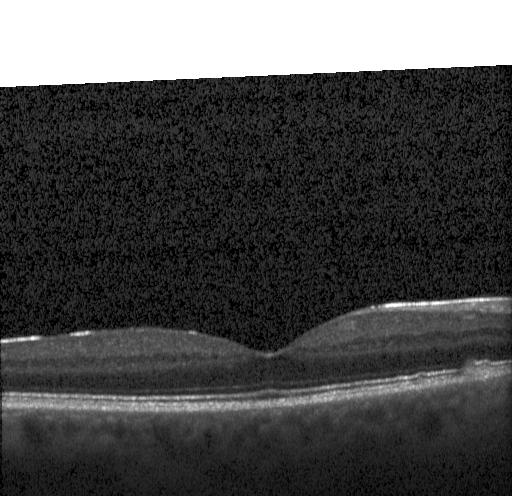

Retinal OCT cross-section.
Impression: sub-RPE drusenoid deposits.